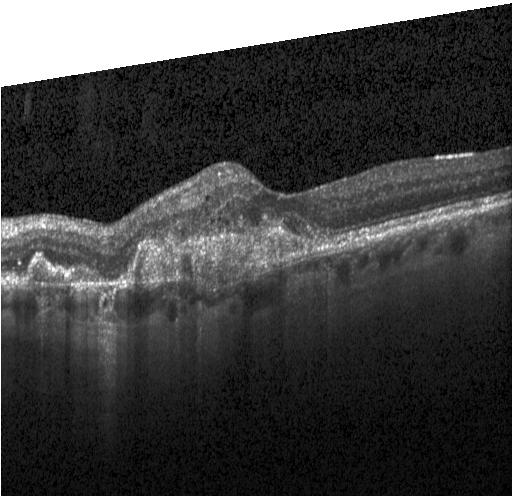
Spectral-domain OCT B-scan: a choroidal neovascular membrane.